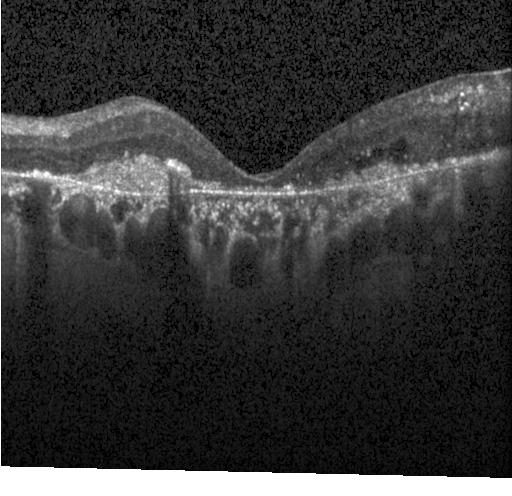
Centered on the fovea · acquired on a Heidelberg Spectralis · optical coherence tomography scan.
A choroidal neovascular membrane.